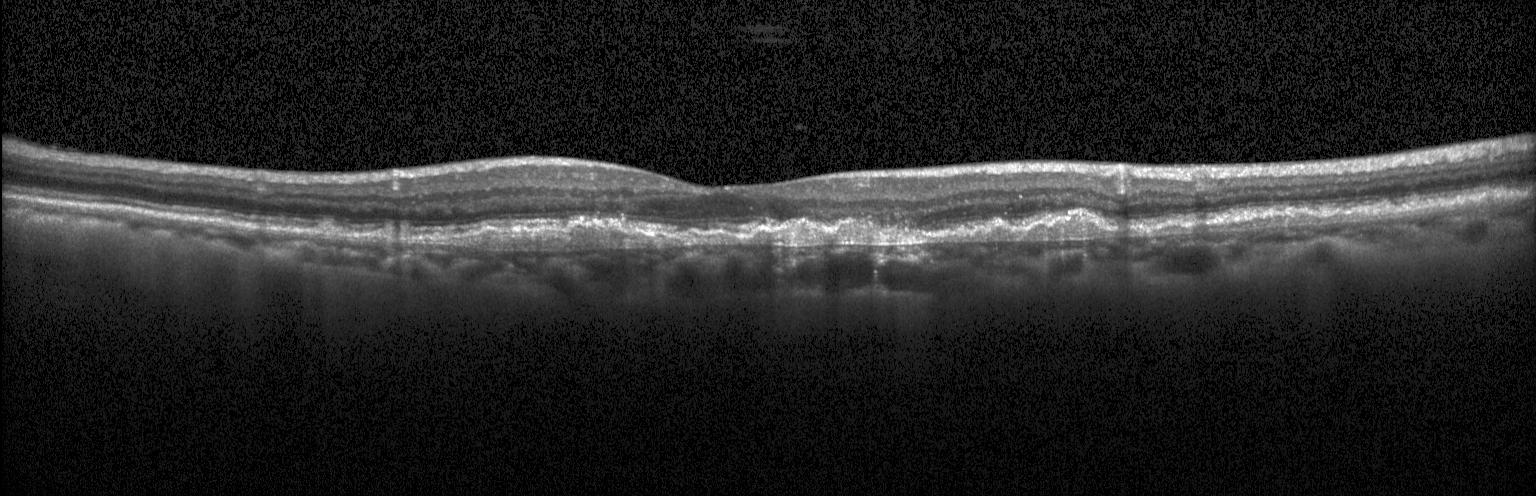 Heidelberg Spectralis · spectral-domain optical coherence tomography · macular scan · retinal OCT B-scan
Assessment: CNV.